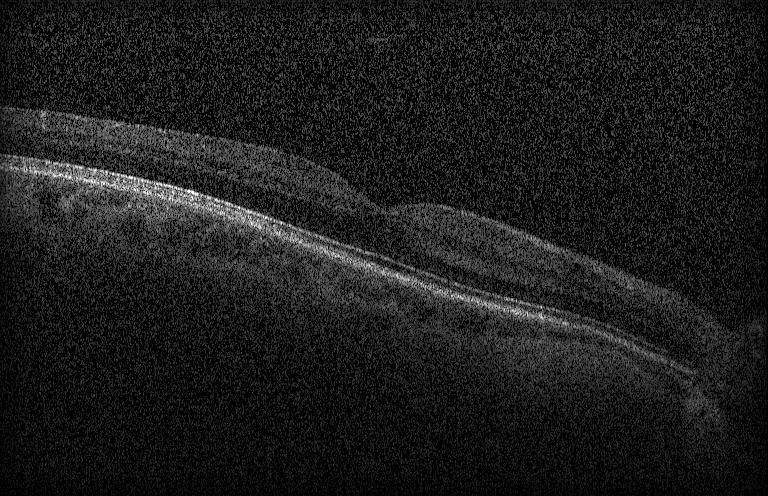

Heidelberg Spectralis OCT system · retinal OCT cross-section.
This B-scan demonstrates no CNV, DME, or drusen.